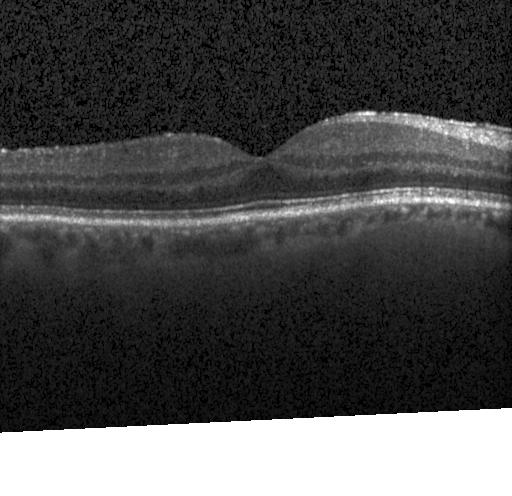 Horizontal scan through the fovea; OCT B-scan; spectral-domain optical coherence tomography — Dx: no CNV, no DME, and no drusen.